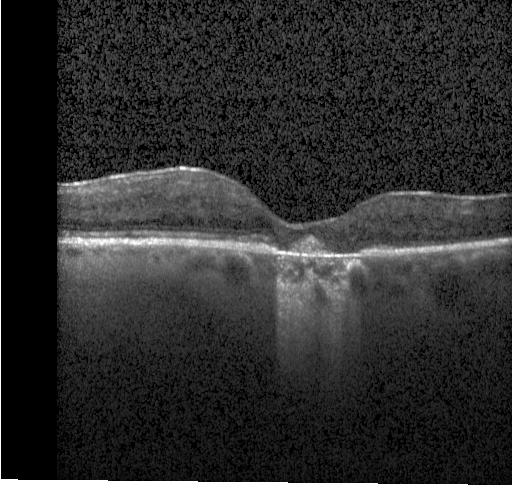
Diagnosis: CNV.